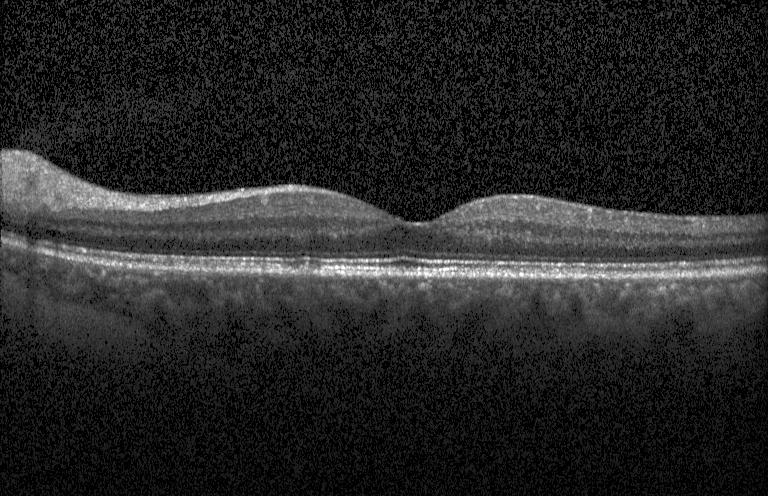 Retinal OCT B-scan. Heidelberg Spectralis OCT system. Diagnosis: no evidence of choroidal neovascularization, diabetic macular edema, or drusen.